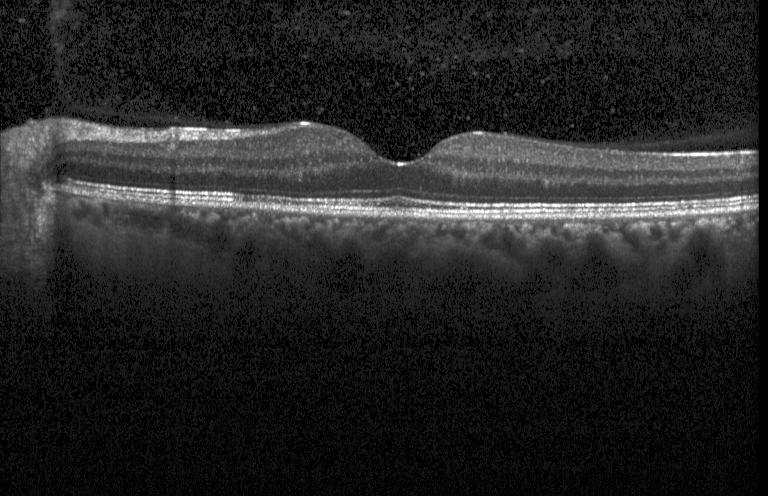

Dx: neither CNV, DME, nor drusen.